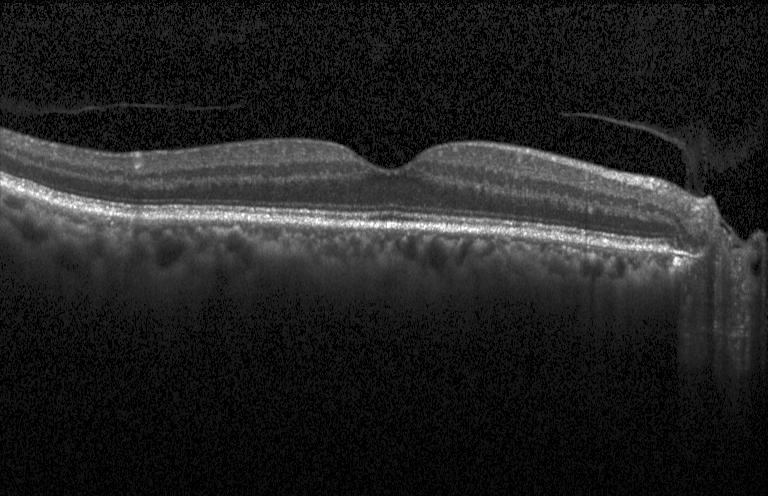 Macular scan · Heidelberg Spectralis · OCT line scan
No choroidal neovascularization, no diabetic macular edema, and no drusen.